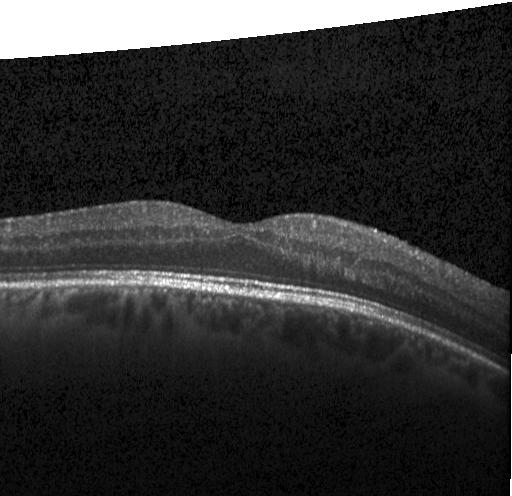 Horizontal scan through the fovea, retinal OCT B-scan.
Diagnosis: no evidence of choroidal neovascularization, diabetic macular edema, or drusen.